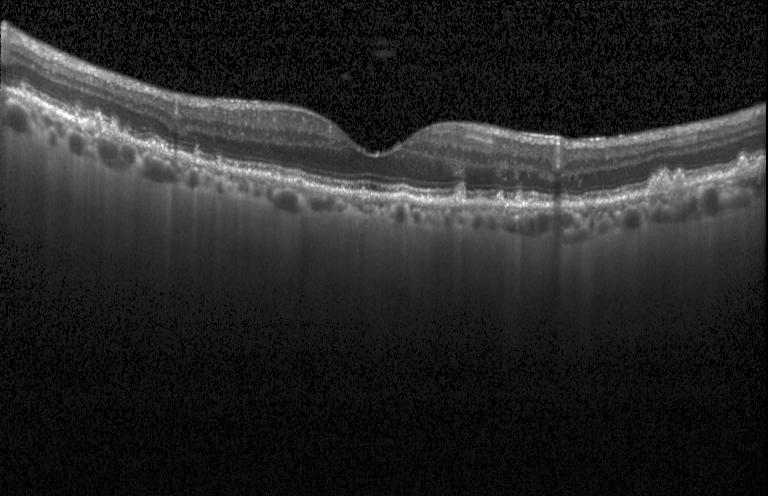
Macular OCT: multiple drusen.